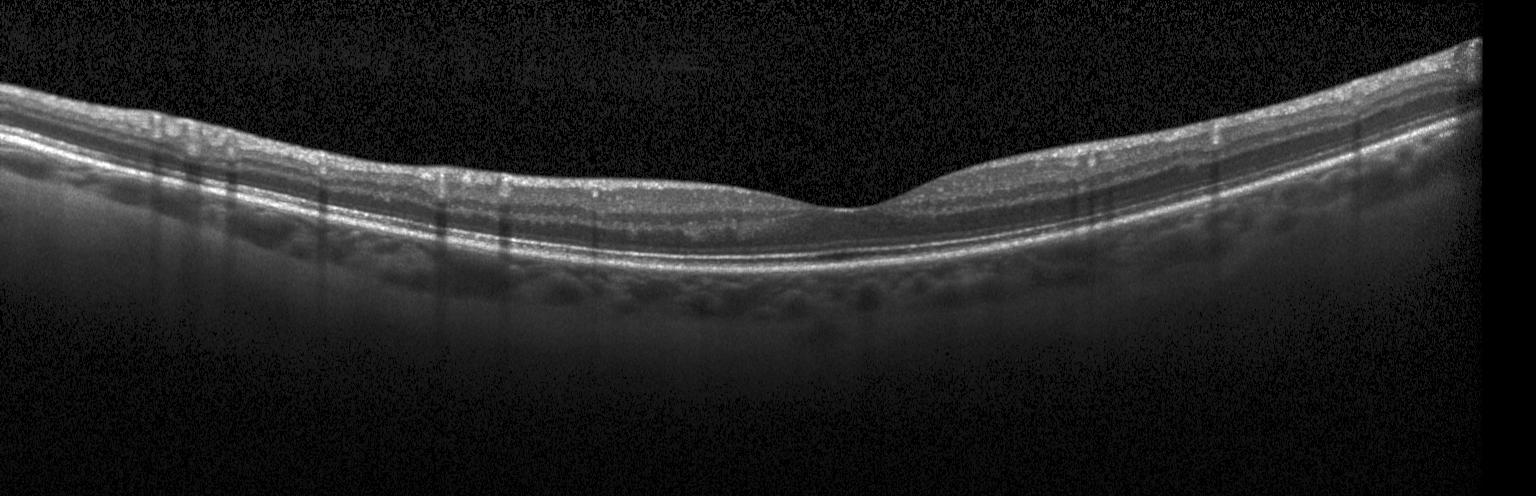

OCT B-scan, SD-OCT, horizontal scan through the fovea, Heidelberg Spectralis — Finding: neither choroidal neovascularization, diabetic macular edema, nor drusen.